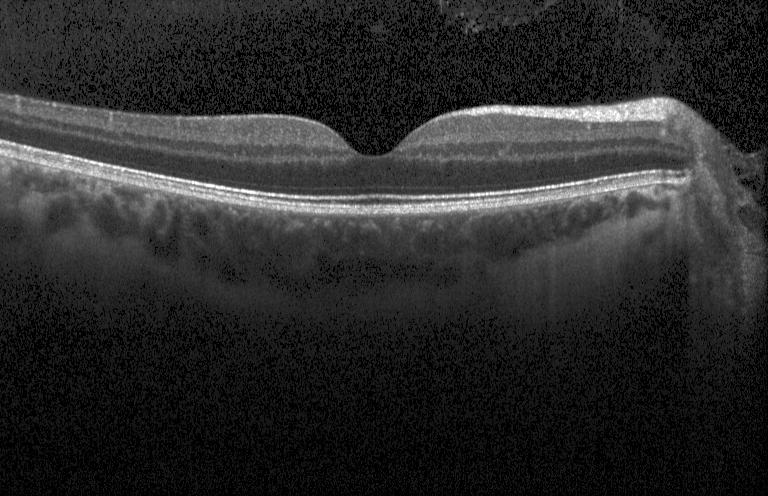 Optical coherence tomography B-scan.
OCT finding: no evidence of choroidal neovascularization, diabetic macular edema, or drusen.